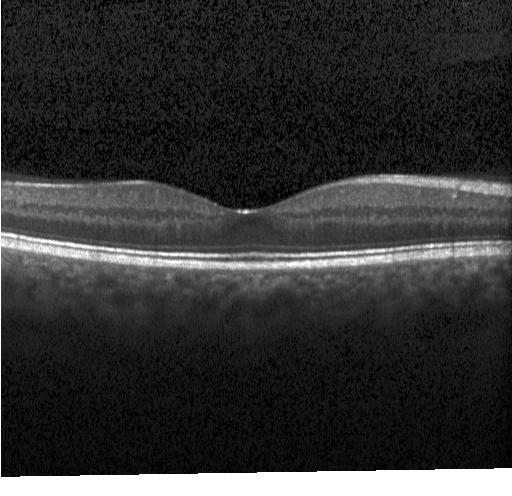
Macular OCT: neither CNV, DME, nor drusen.